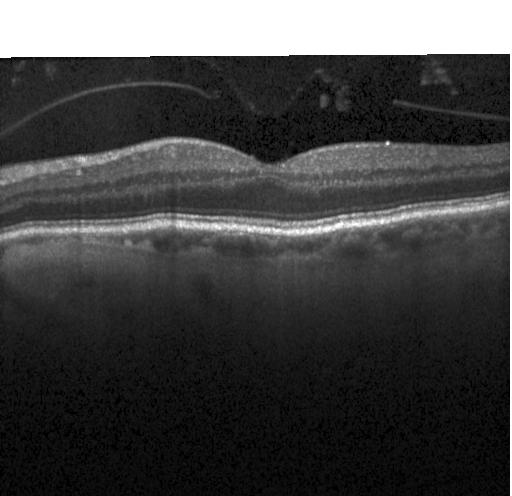 Heidelberg Spectralis OCT system · fovea-centered · retinal OCT cross-section.
This B-scan demonstrates no choroidal neovascularization, no diabetic macular edema, and no drusen.